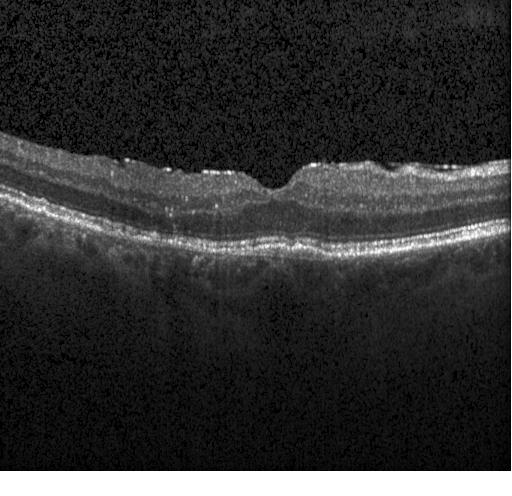 Acquired on a Heidelberg Spectralis. Optical coherence tomography B-scan
This B-scan demonstrates a choroidal neovascular membrane.